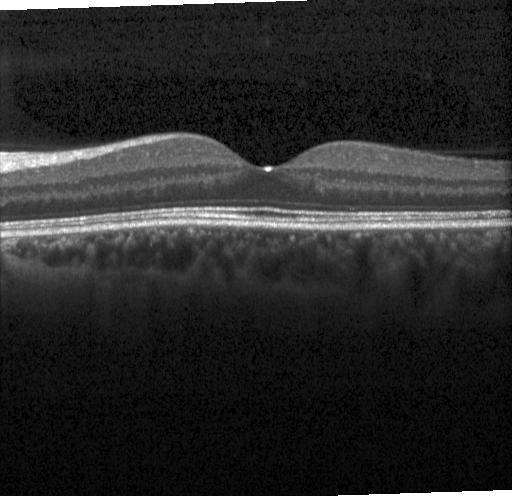 Optical coherence tomography scan, spectral-domain OCT
Finding: neither choroidal neovascularization, diabetic macular edema, nor drusen.